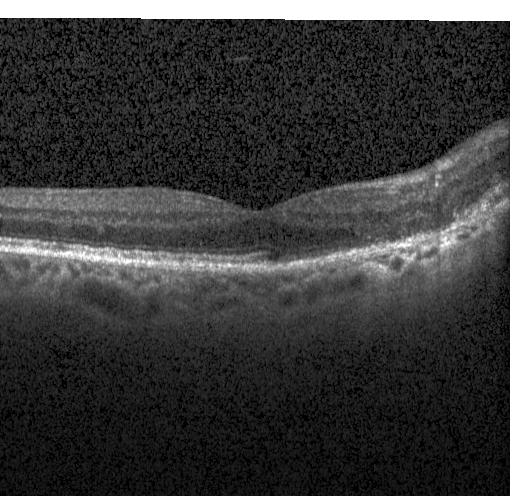

OCT line scan. Through the macula. Assessment: choroidal neovascularization.